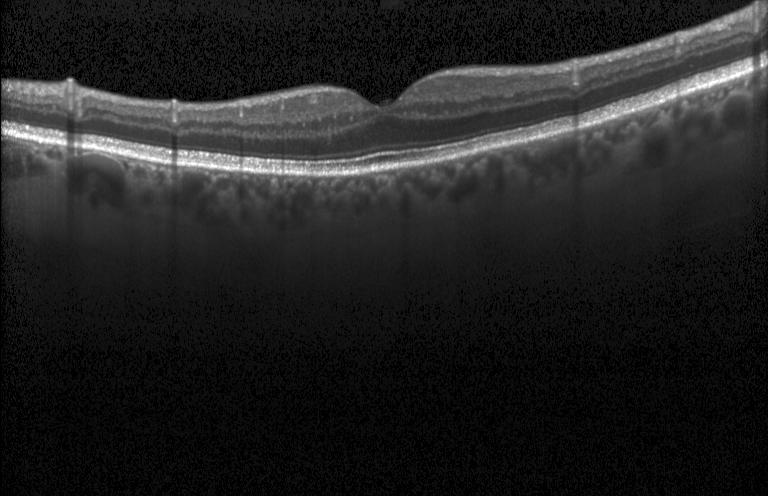 Acquired on a Heidelberg Spectralis. OCT line scan
Assessment: no CNV, no DME, and no drusen.